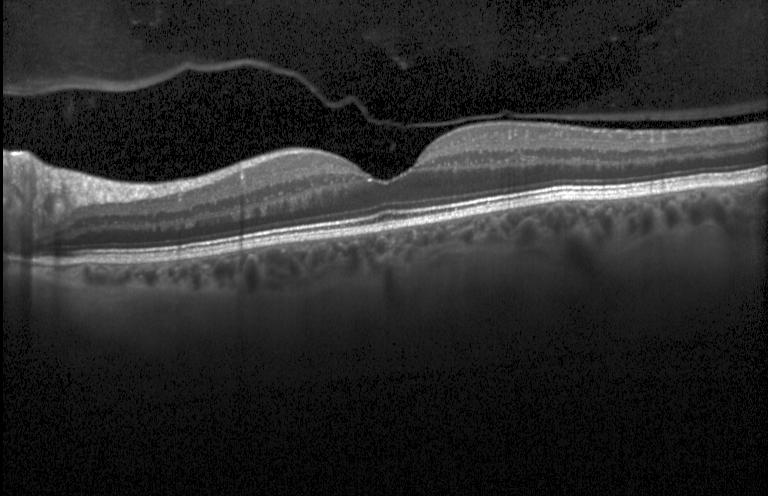
Finding: neither choroidal neovascularization, diabetic macular edema, nor drusen.